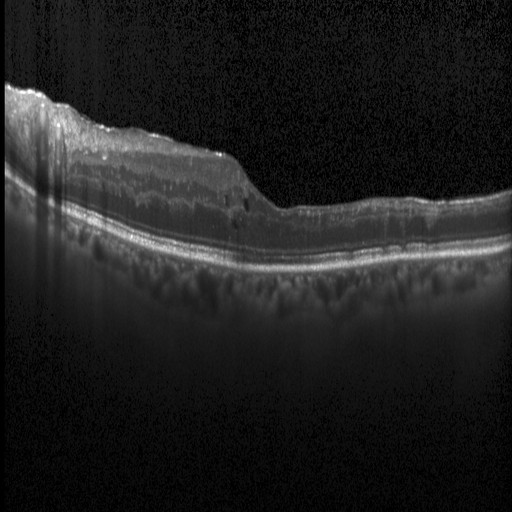
Diagnosis: DME.